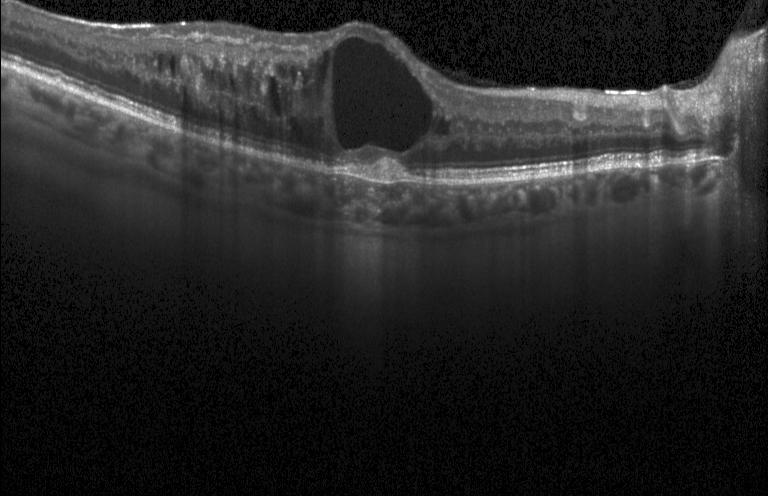

Retinal OCT B-scan, SD-OCT, Heidelberg Spectralis — Finding: choroidal neovascularization (CNV).